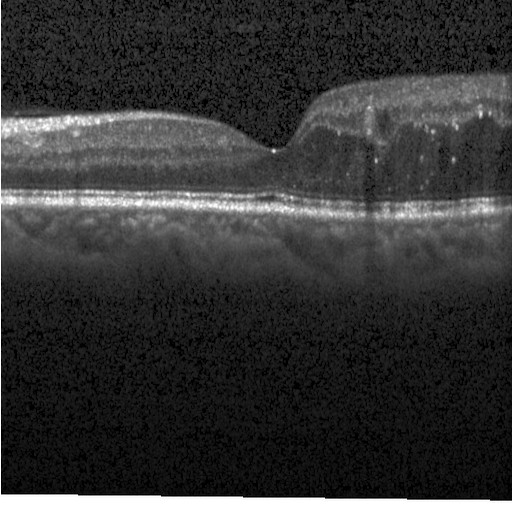
Impression: diabetic macular edema (DME).